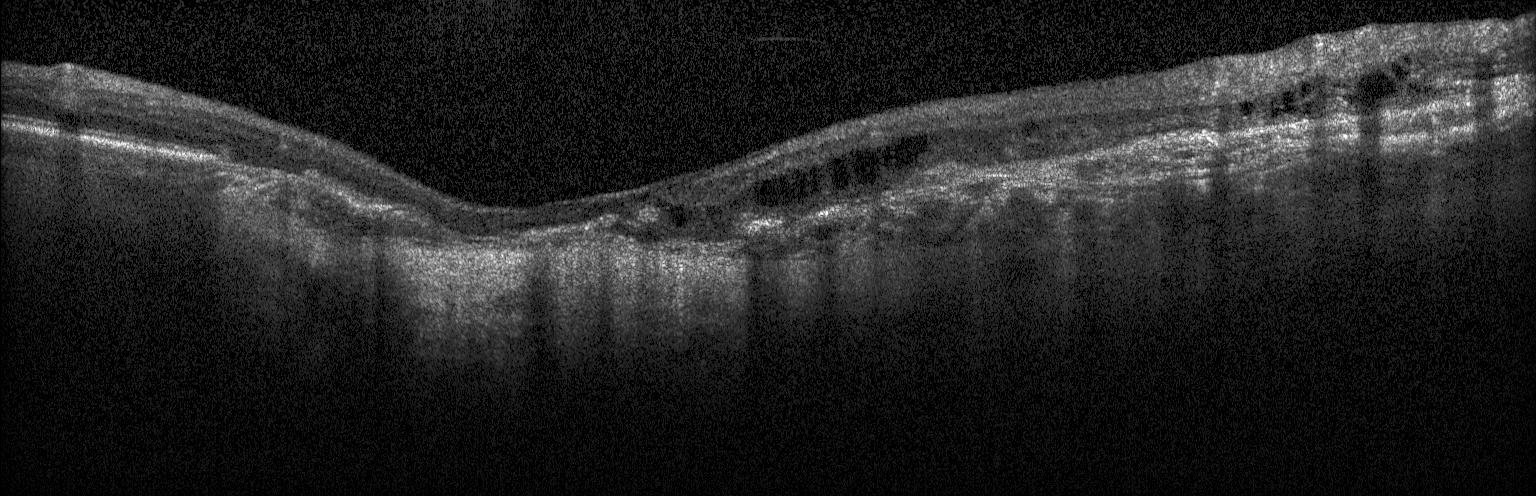

Impression: choroidal neovascularization.